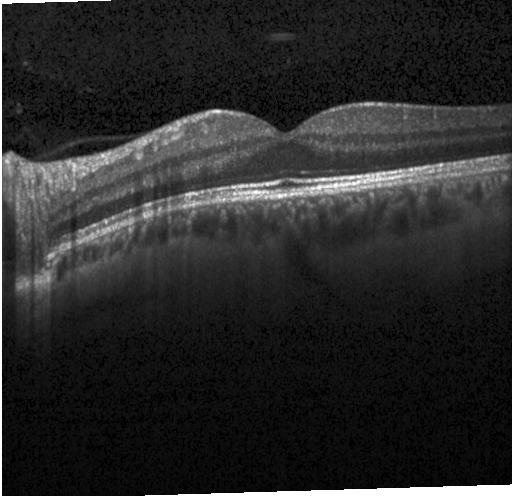
Fovea-centered; optical coherence tomography B-scan; SD-OCT.
Macular OCT: no choroidal neovascularization, no diabetic macular edema, and no drusen.